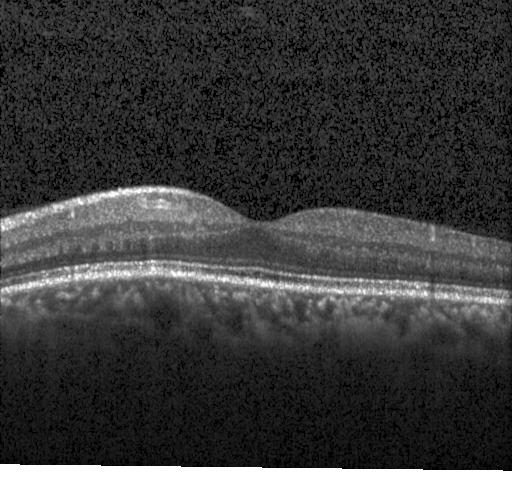

Spectral-domain OCT B-scan: no CNV, no DME, and no drusen.